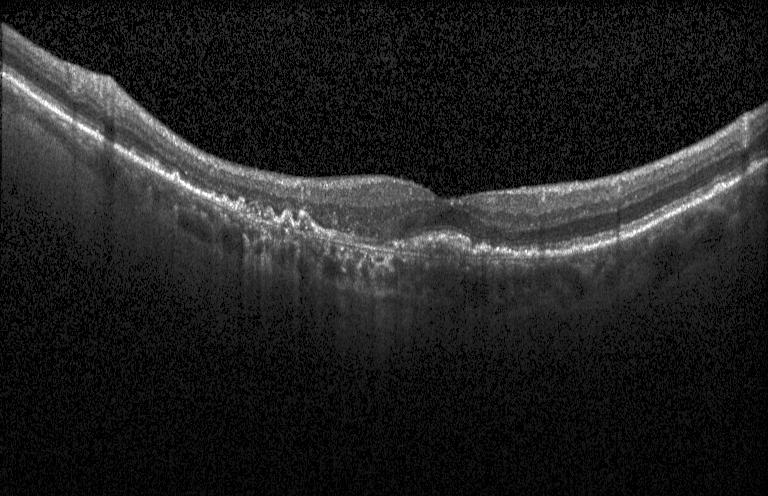 Retinal OCT B-scan — Impression: choroidal neovascularization.